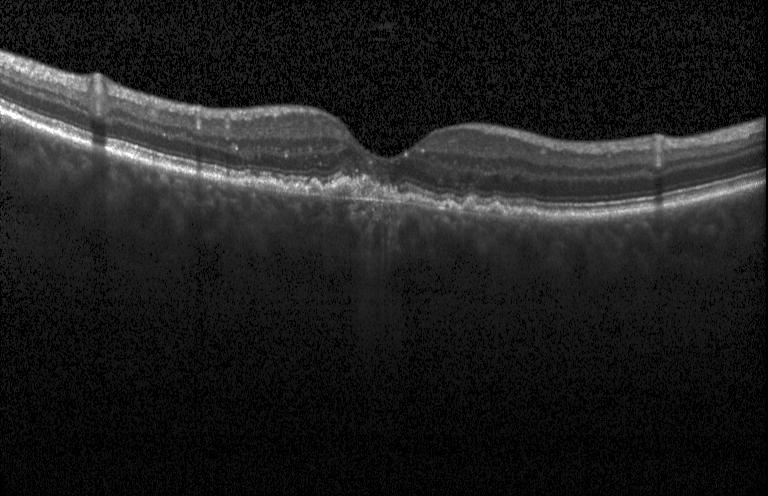 Assessment: choroidal neovascularization.